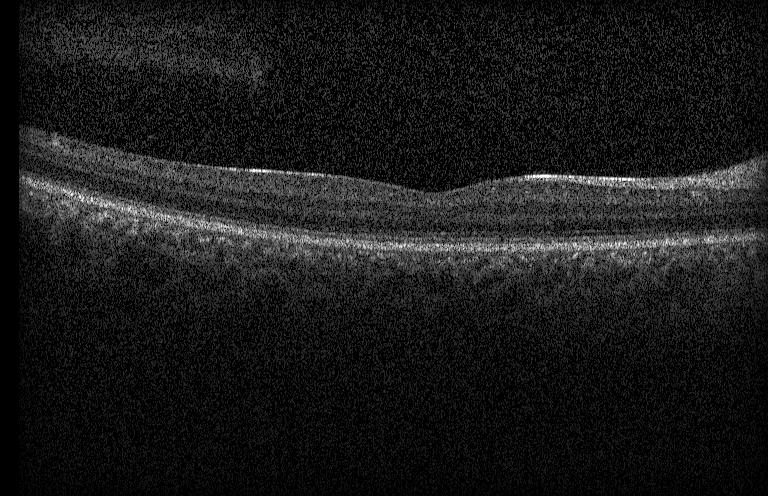
Finding: no choroidal neovascularization, no diabetic macular edema, and no drusen.